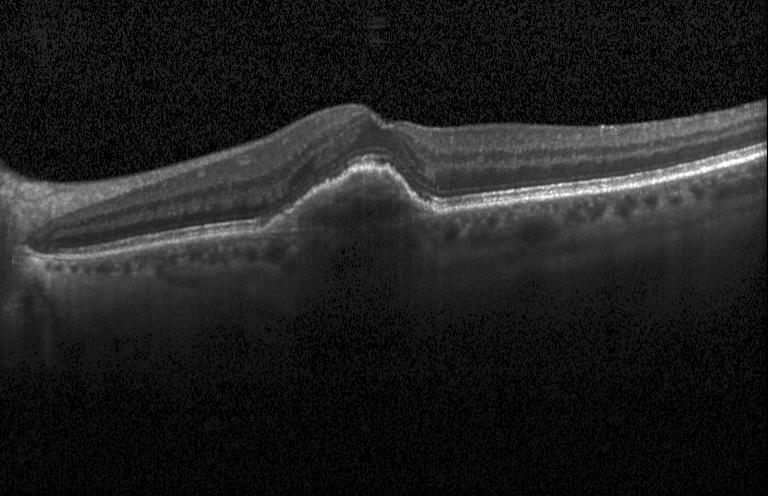
OCT B-scan
Dx: a choroidal neovascular membrane.